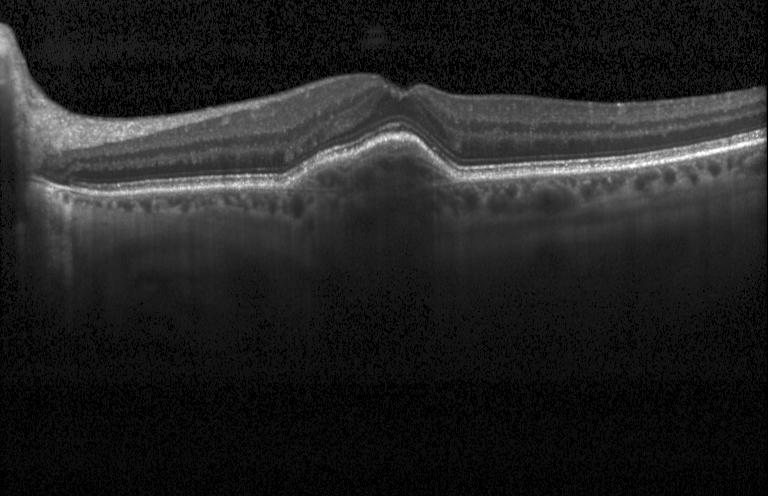 Through the macula, optical coherence tomography B-scan.
Finding: choroidal neovascularization.